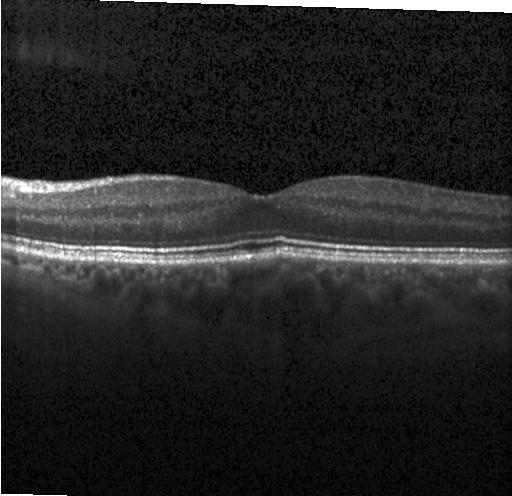

Heidelberg Spectralis · OCT line scan. Assessment: no evidence of CNV, DME, or drusen.